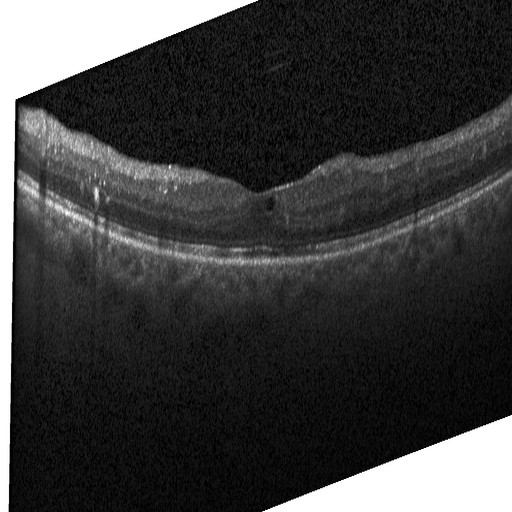
Macular OCT: DME.